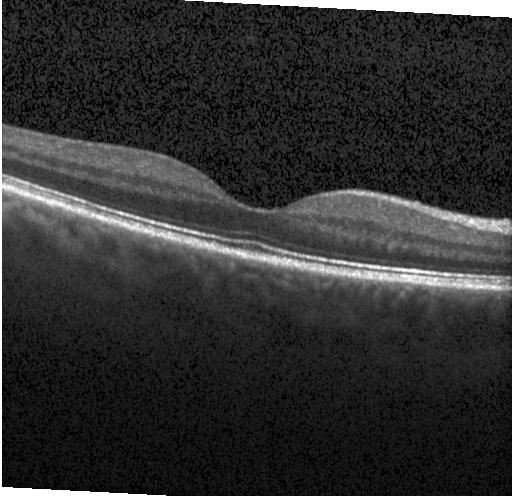

SD-OCT · retinal OCT cross-section. Assessment: no evidence of CNV, DME, or drusen.